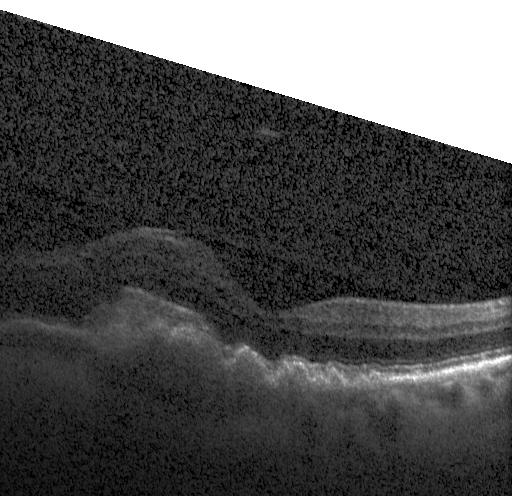

Finding: choroidal neovascularization.